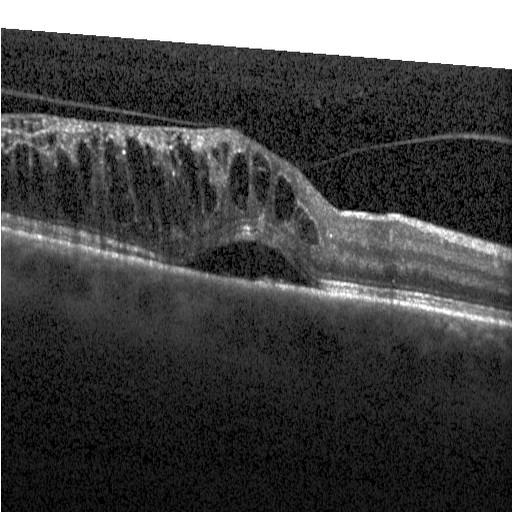

Diagnosis: diabetic macular edema (DME).